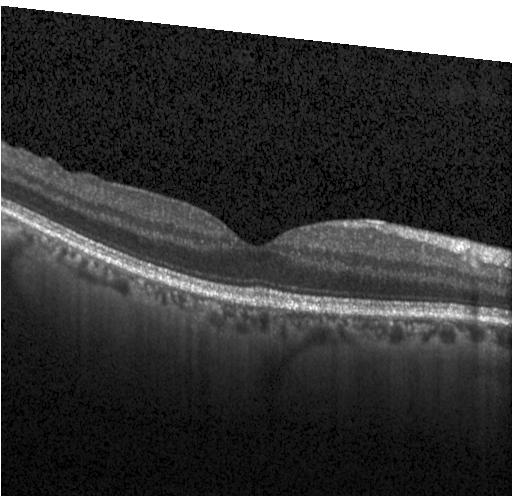
OCT line scan
Finding: no evidence of choroidal neovascularization, diabetic macular edema, or drusen.